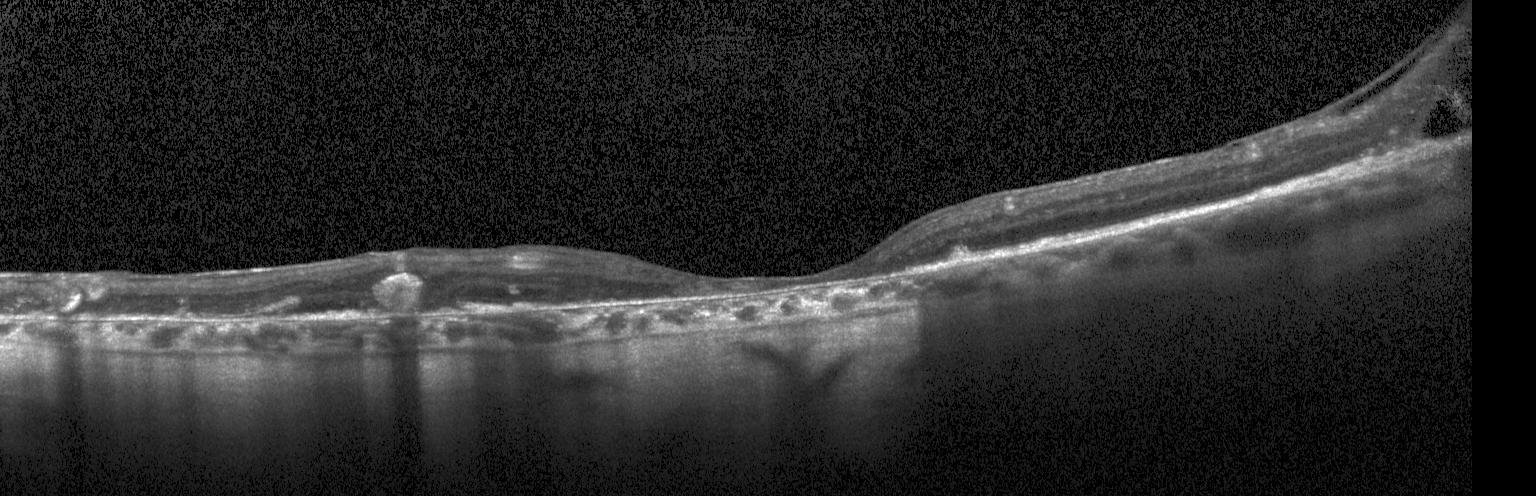

Diagnosis: CNV.